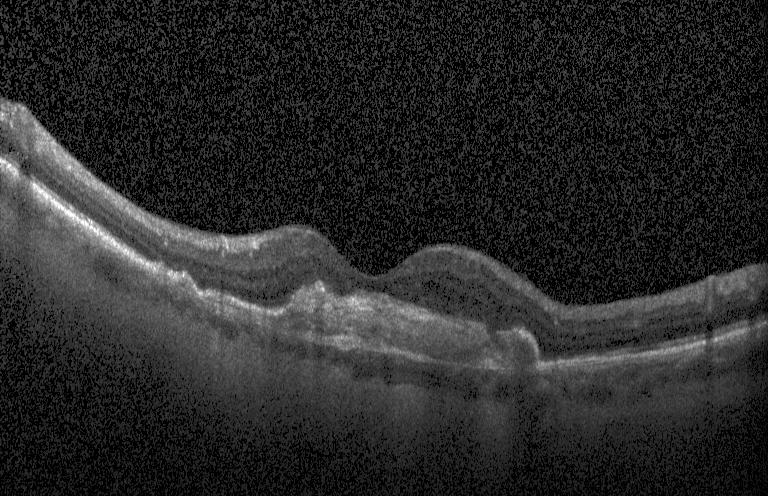

Optical coherence tomography B-scan. Assessment: a choroidal neovascular membrane.